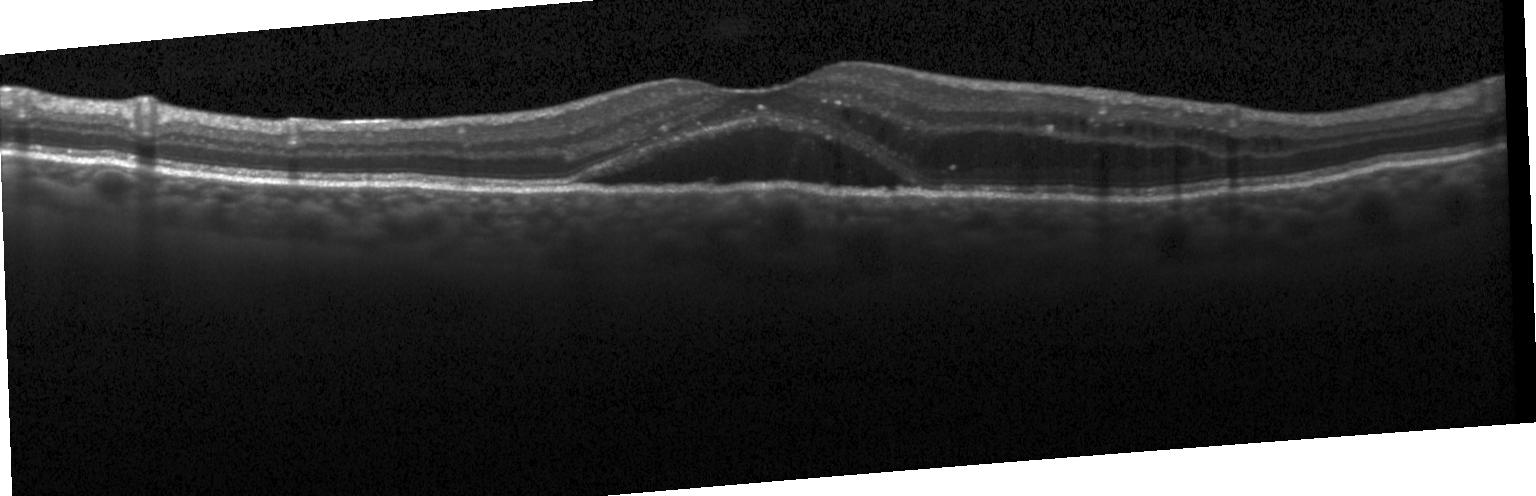
Heidelberg Spectralis · retinal OCT B-scan · through the macula. This B-scan demonstrates diabetic macular edema (DME).